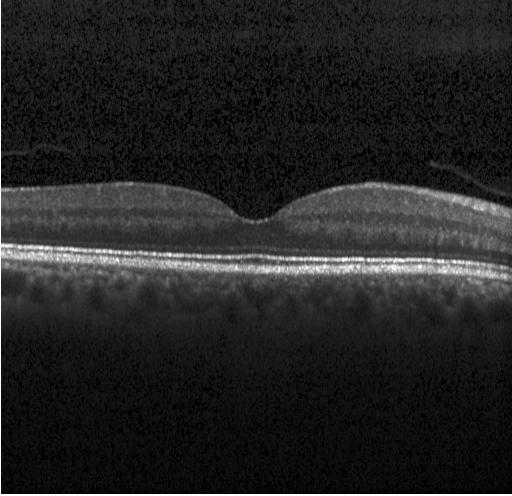 Instrument: Heidelberg Spectralis · OCT B-scan.
The scan shows no CNV, DME, or drusen.